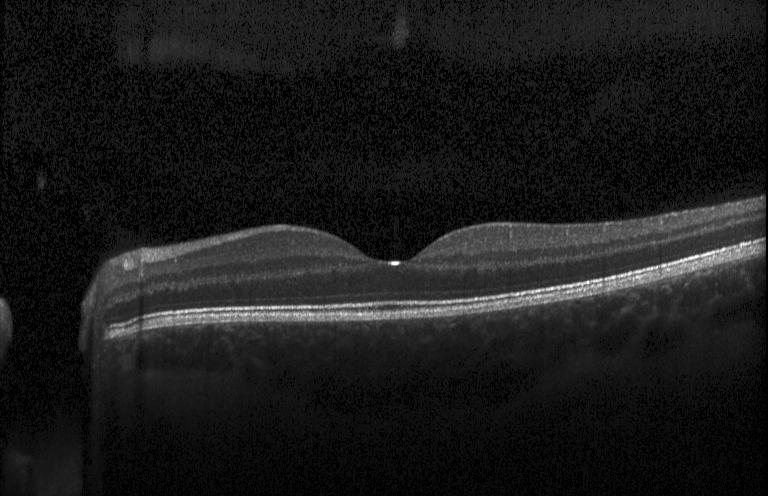

Retinal OCT cross-section showing no choroidal neovascularization, diabetic macular edema, or drusen.